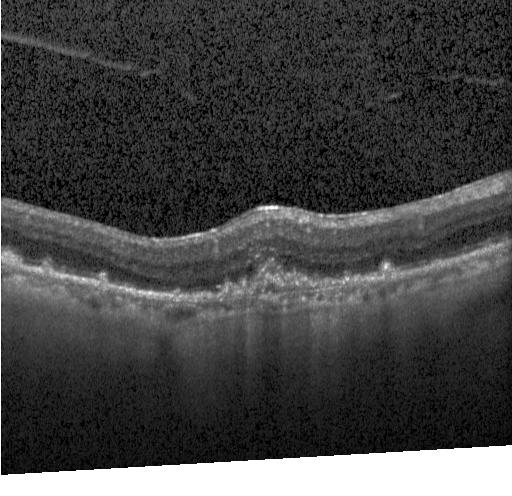

OCT B-scan.
The scan shows a choroidal neovascular membrane.